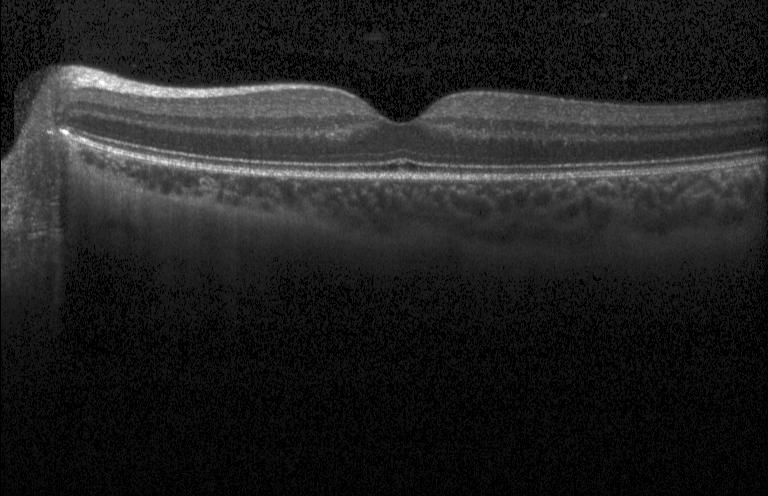 Diagnosis: no choroidal neovascularization, no diabetic macular edema, and no drusen.